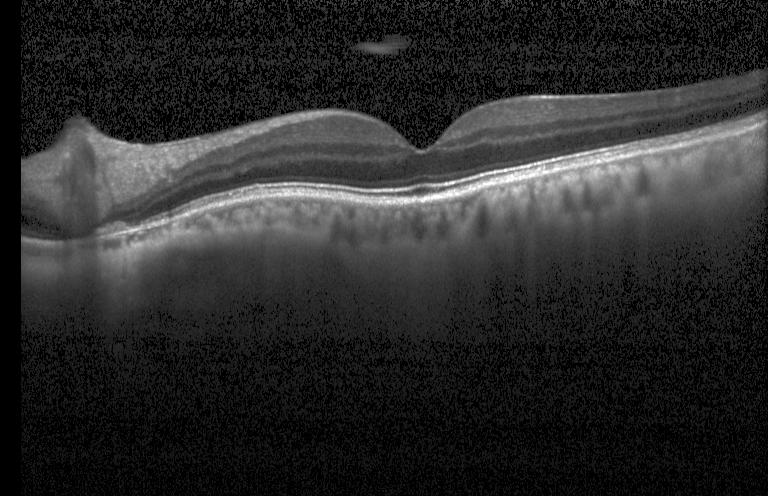
Optical coherence tomography scan. SD-OCT. Fovea-centered. Instrument: Heidelberg Spectralis — Finding: neither choroidal neovascularization, diabetic macular edema, nor drusen.